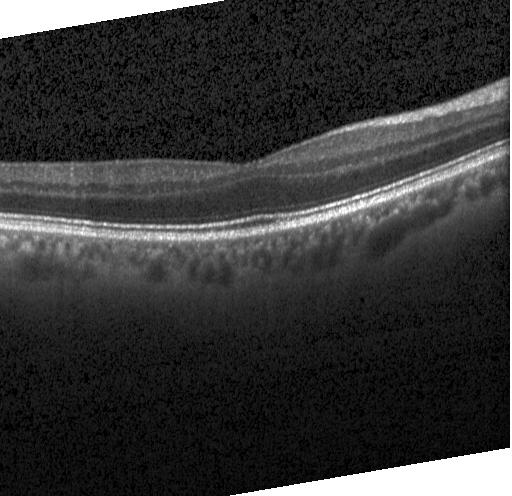

SD-OCT; horizontal scan through the fovea; OCT B-scan.
Dx: neither CNV, DME, nor drusen.